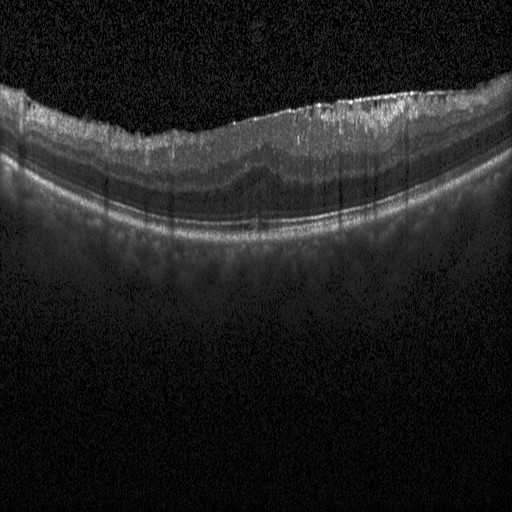

The scan shows diabetic macular edema.